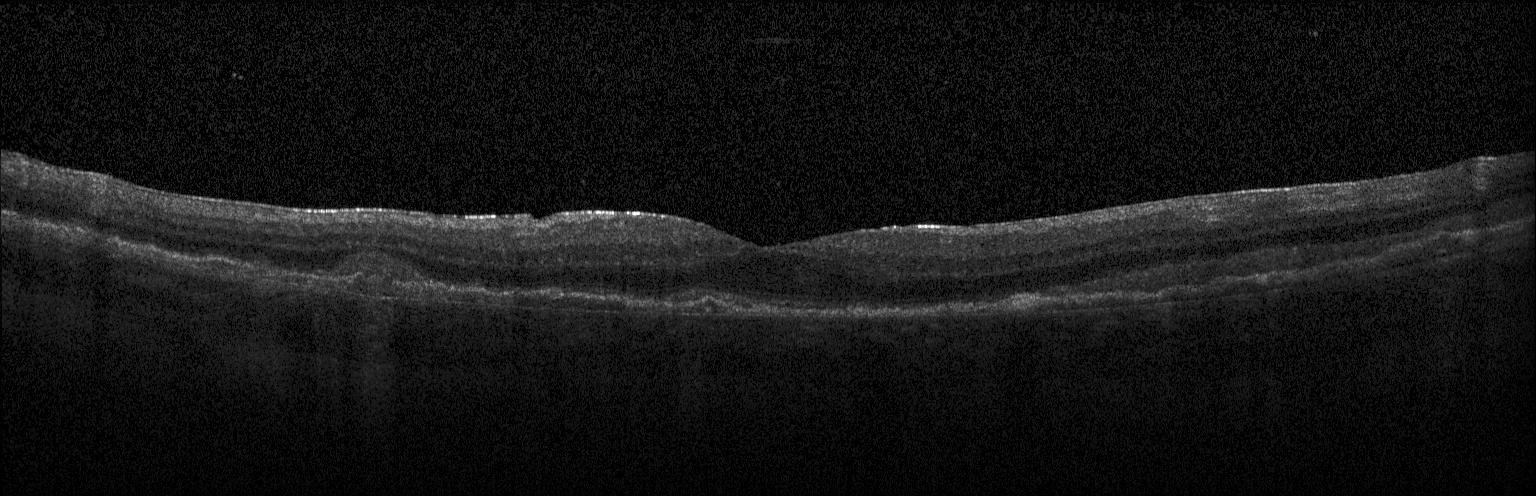

Optical coherence tomography scan.
Assessment: a choroidal neovascular membrane.